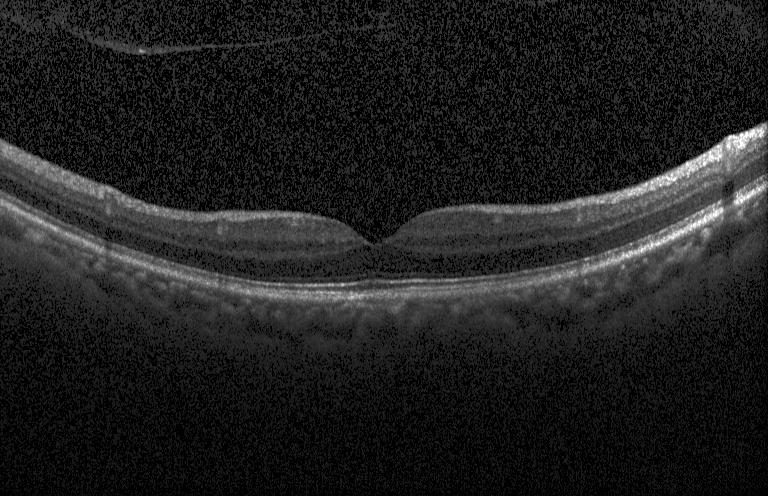 Optical coherence tomography B-scan; instrument: Heidelberg Spectralis
Diagnosis: no choroidal neovascularization, no diabetic macular edema, and no drusen.